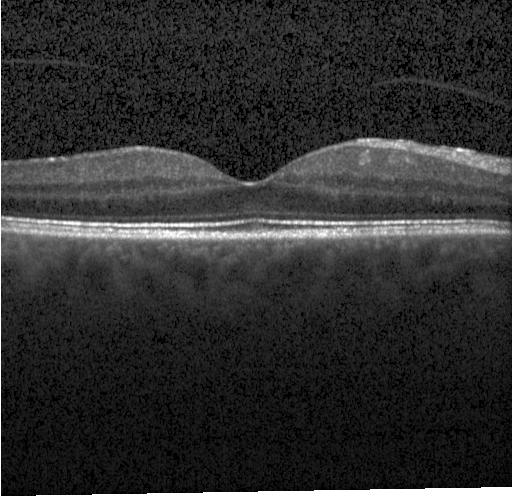
Finding: no CNV, no DME, and no drusen.